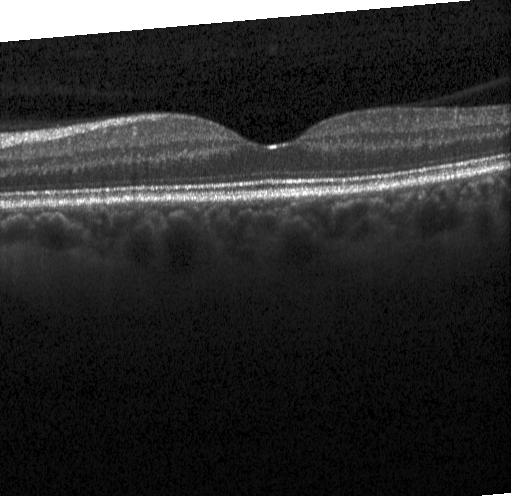 Finding: neither choroidal neovascularization, diabetic macular edema, nor drusen.